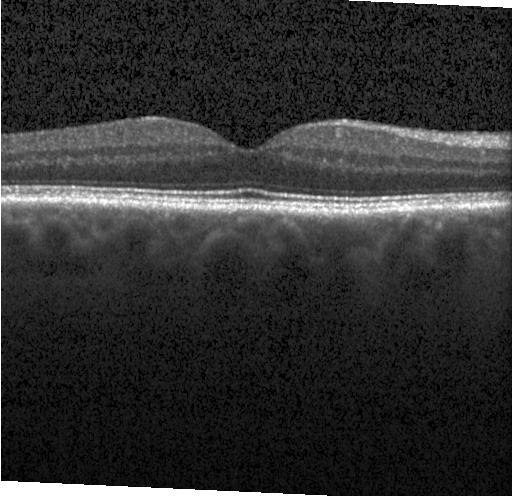
OCT line scan. Macular scan. Instrument: Heidelberg Spectralis.
This B-scan demonstrates no choroidal neovascularization, diabetic macular edema, or drusen.